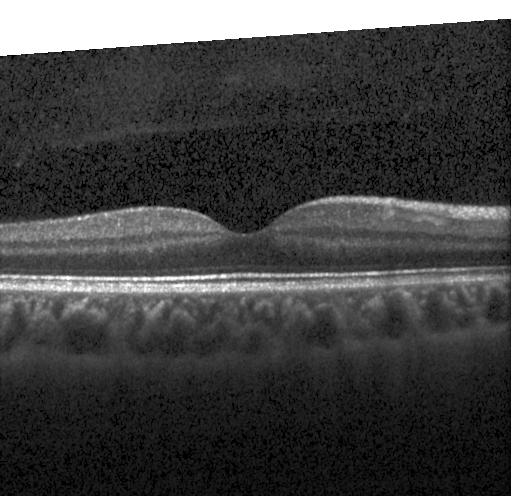
Spectral-domain OCT; retinal OCT cross-section — Assessment: no evidence of CNV, DME, or drusen.